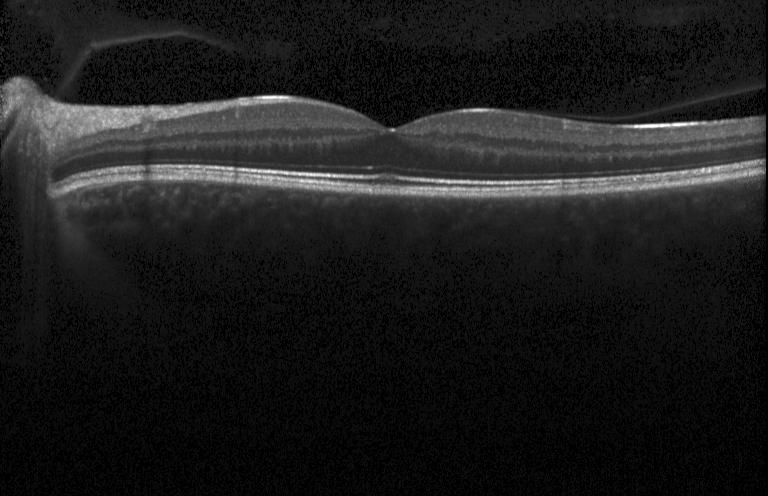 OCT line scan. SD-OCT — No choroidal neovascularization, no diabetic macular edema, and no drusen.